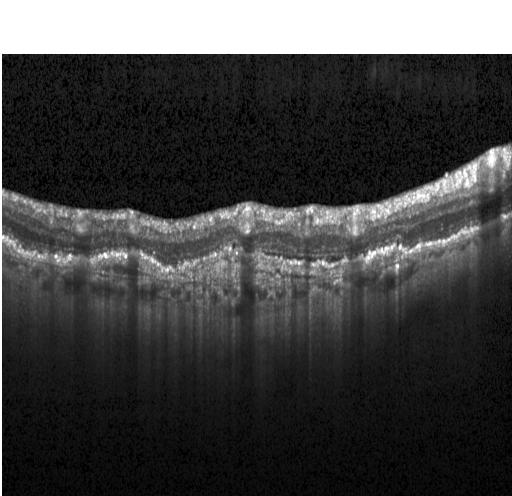
Spectral-domain optical coherence tomography. Horizontal scan through the fovea. Retinal OCT cross-section. Heidelberg Spectralis OCT system. Diagnosis: a choroidal neovascular membrane.